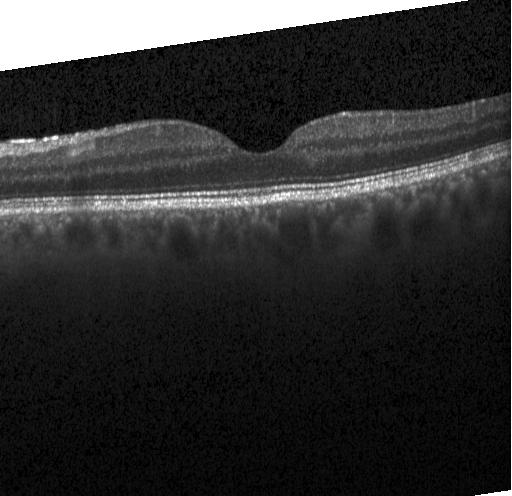

Assessment: neither CNV, DME, nor drusen.